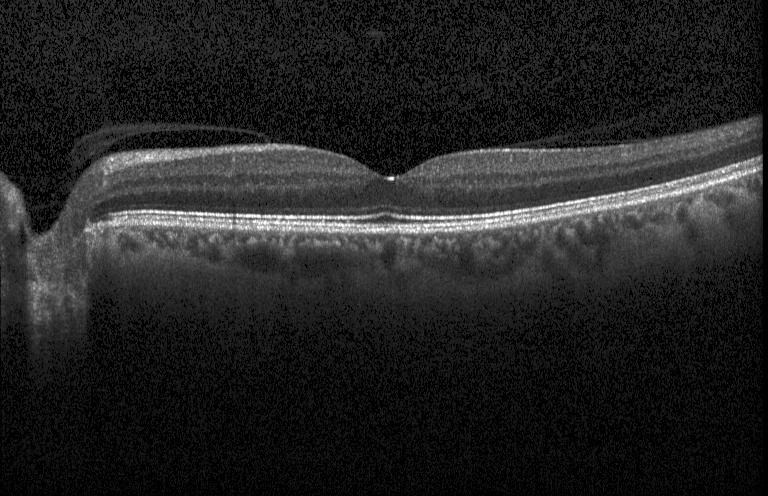 Impression: no evidence of CNV, DME, or drusen.